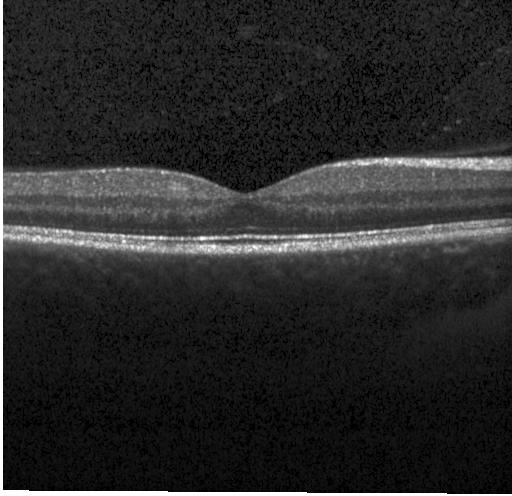 Macular OCT: no evidence of CNV, DME, or drusen.